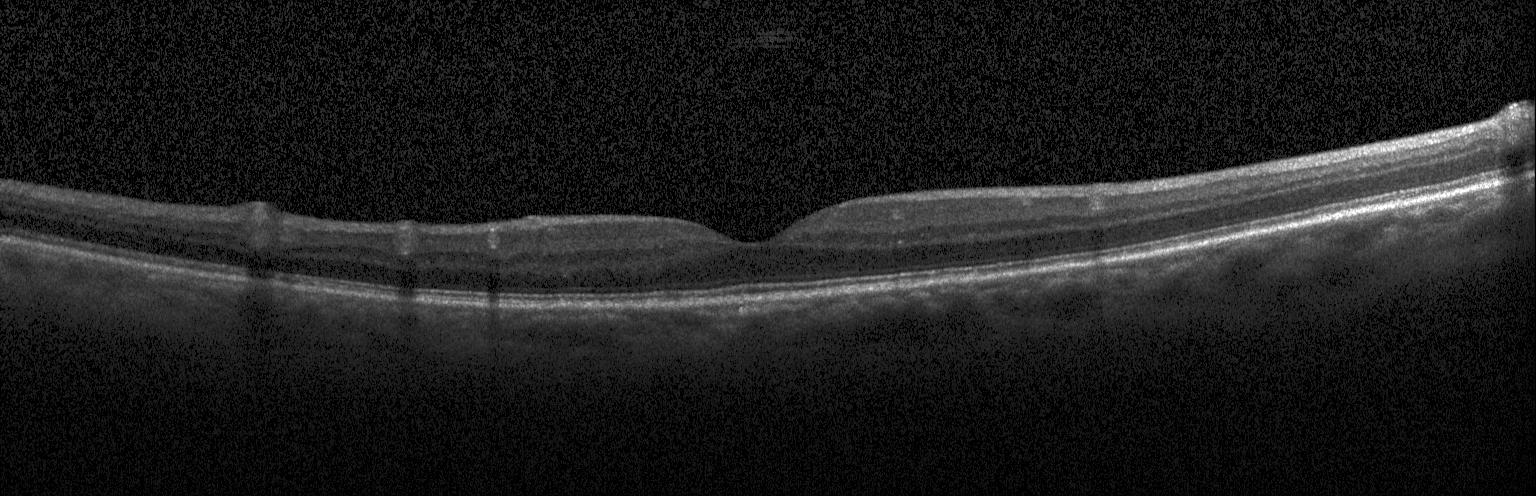 Retinal OCT B-scan. Macular OCT: neither CNV, DME, nor drusen.